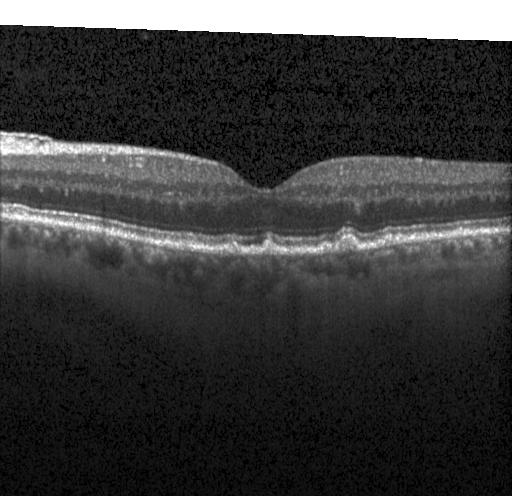 OCT finding: multiple drusen.